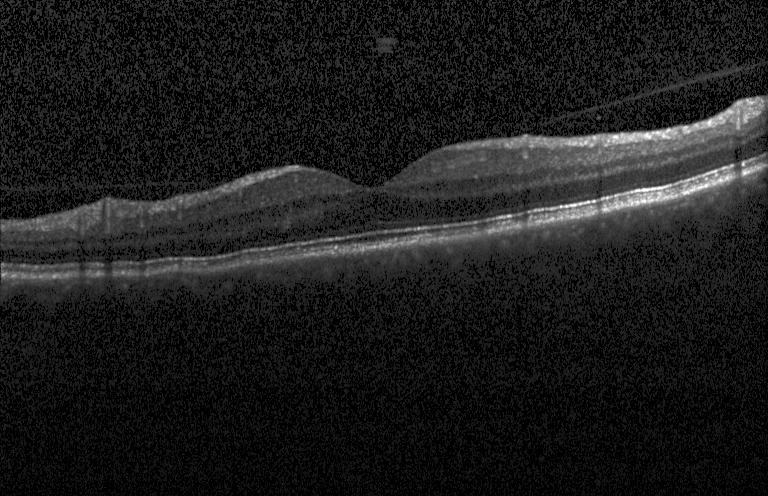
Optical coherence tomography scan · spectral-domain optical coherence tomography
Finding: neither choroidal neovascularization, diabetic macular edema, nor drusen.